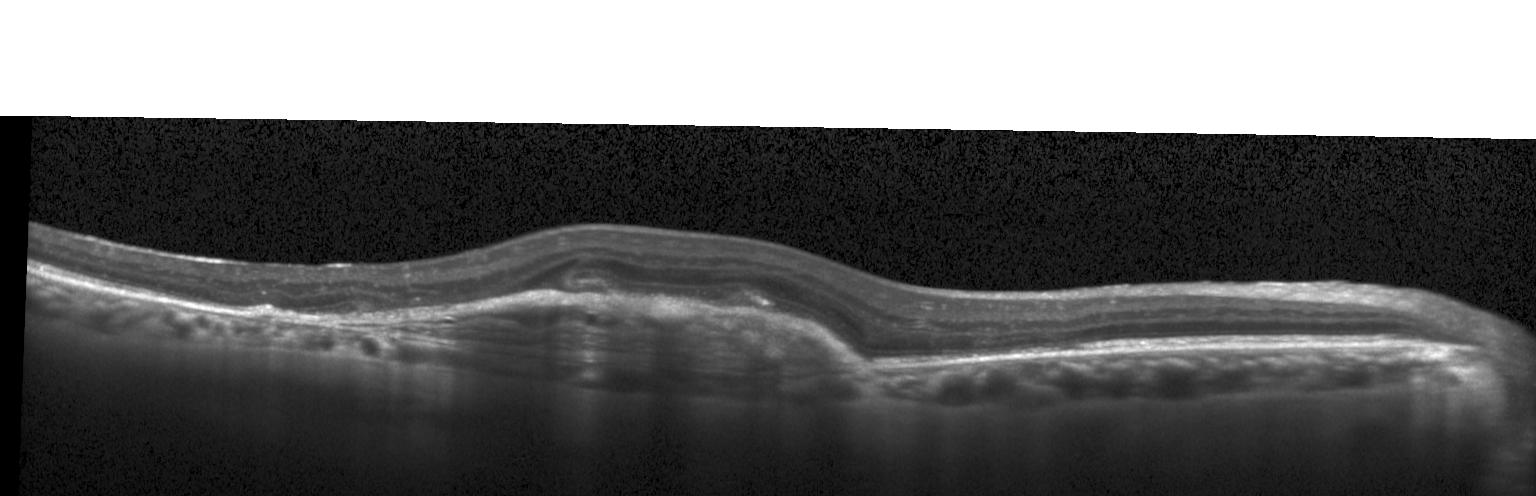
Diagnosis: a choroidal neovascular membrane.